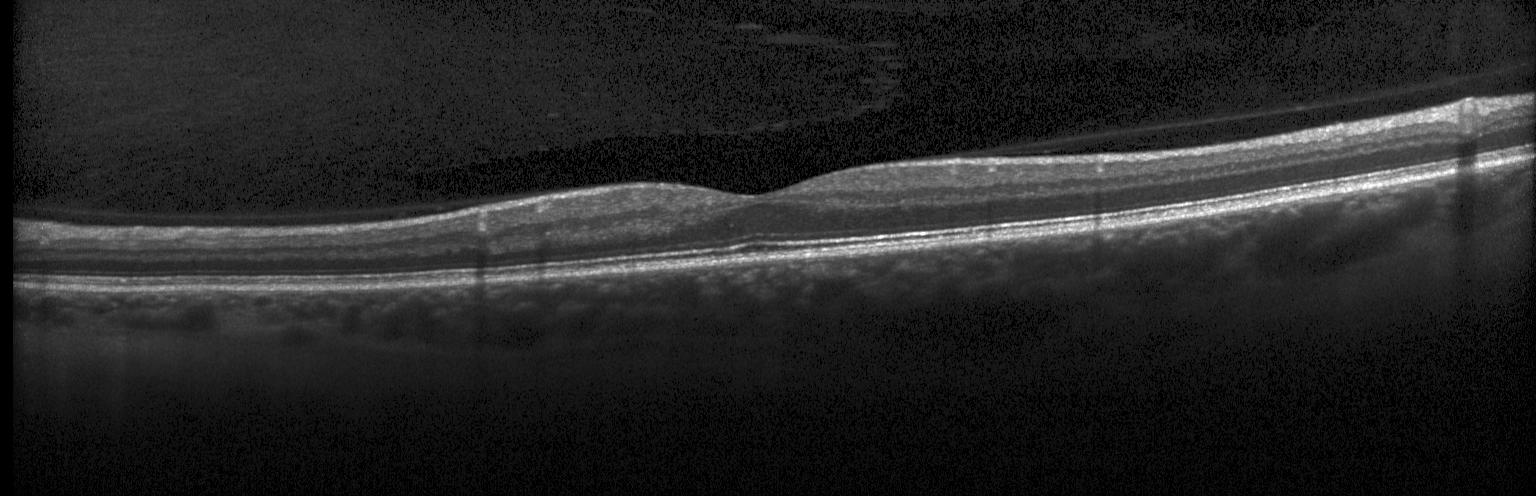 OCT line scan · Heidelberg Spectralis — This B-scan demonstrates no evidence of CNV, DME, or drusen.